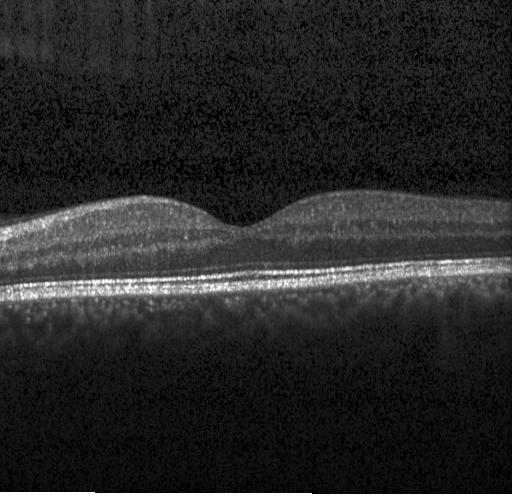 OCT B-scan; fovea-centered — Impression: no CNV, DME, or drusen.